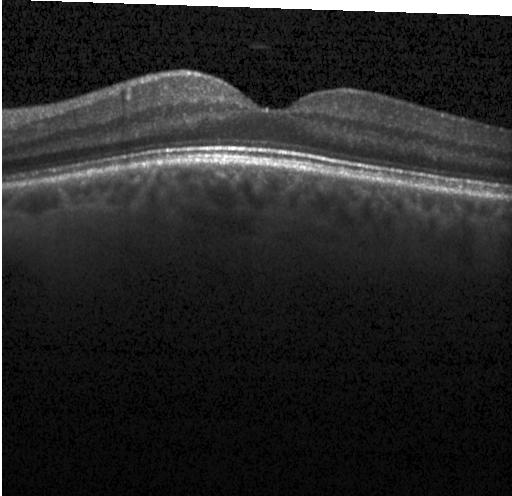 Heidelberg Spectralis; SD-OCT; optical coherence tomography scan; centered on the fovea.
Macular OCT: no CNV, DME, or drusen.